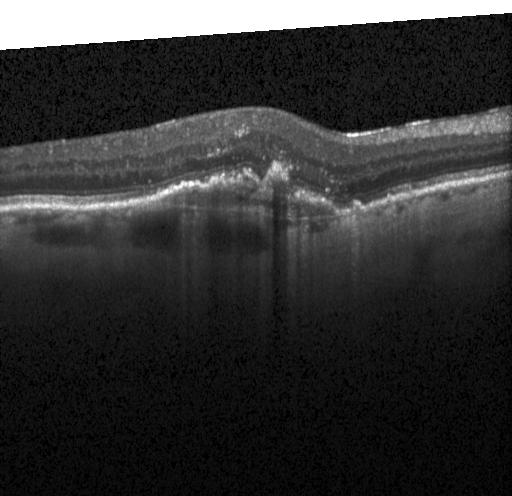
The scan shows CNV.